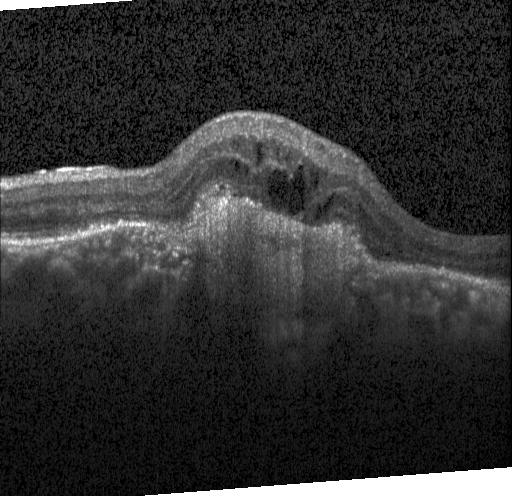 Macular OCT: CNV.